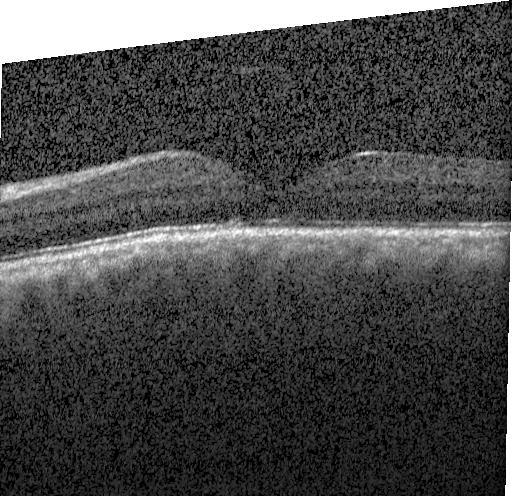

Finding: no CNV, no DME, and no drusen.